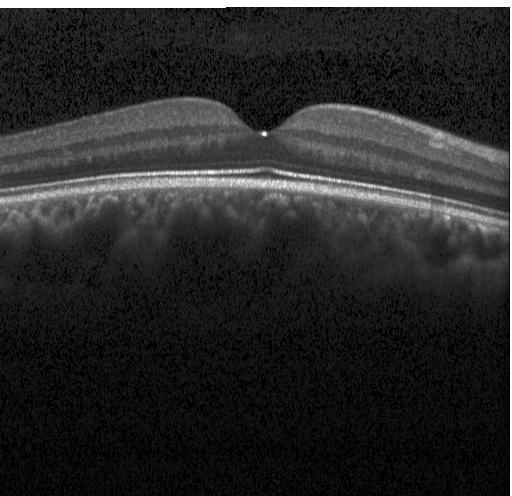
Diagnosis: no CNV, DME, or drusen.